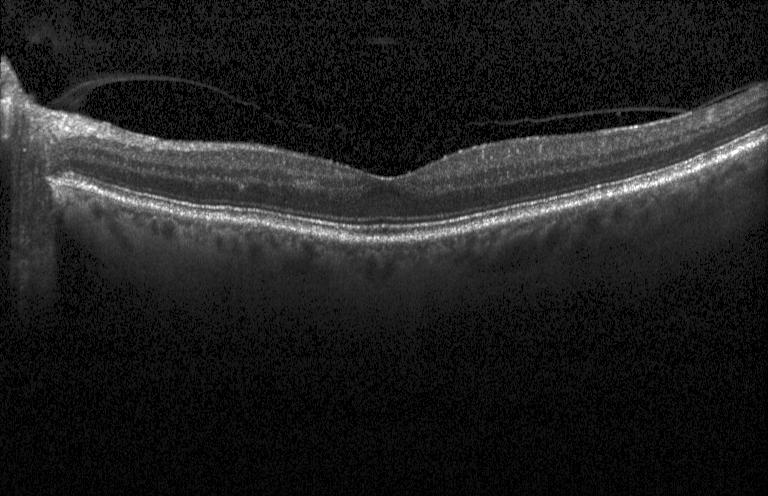 This B-scan demonstrates no choroidal neovascularization, diabetic macular edema, or drusen.